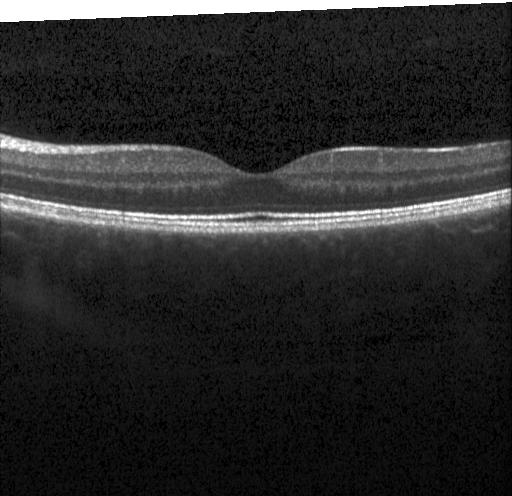 Instrument: Heidelberg Spectralis, horizontal scan through the fovea, retinal OCT B-scan, spectral-domain OCT — Macular OCT: no choroidal neovascularization, no diabetic macular edema, and no drusen.